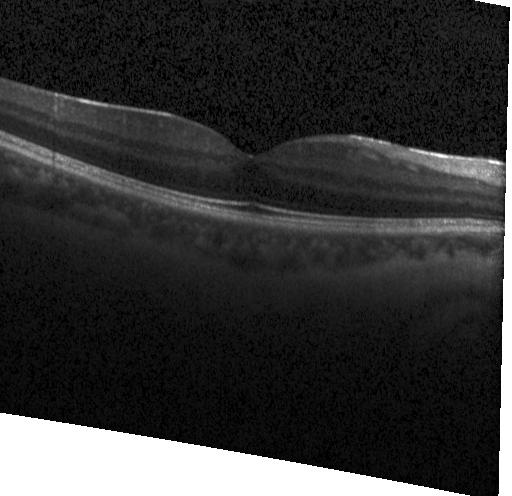 OCT B-scan. Centered on the fovea. Spectral-domain OCT. Acquired on a Heidelberg Spectralis. Diagnosis: no evidence of CNV, DME, or drusen.